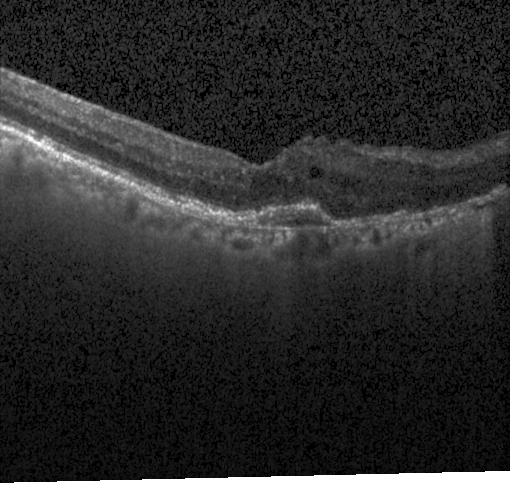
OCT B-scan · instrument: Heidelberg Spectralis · SD-OCT — Dx: choroidal neovascularization.